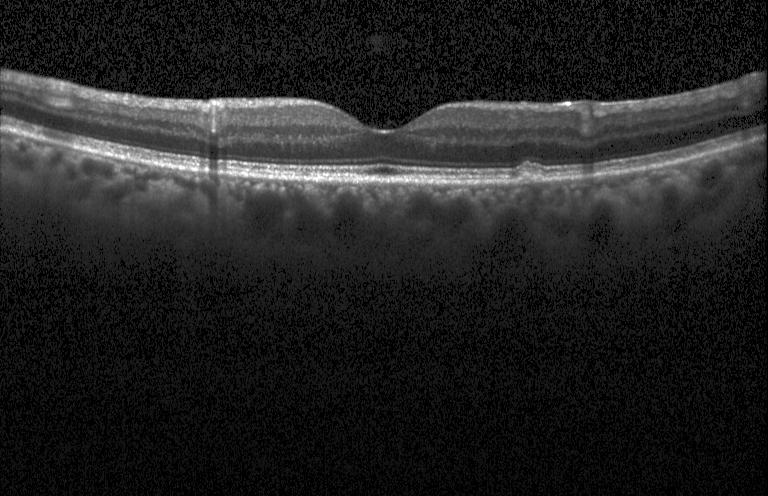 Retinal OCT B-scan, spectral-domain OCT, macular scan, instrument: Heidelberg Spectralis — Impression: multiple drusen.